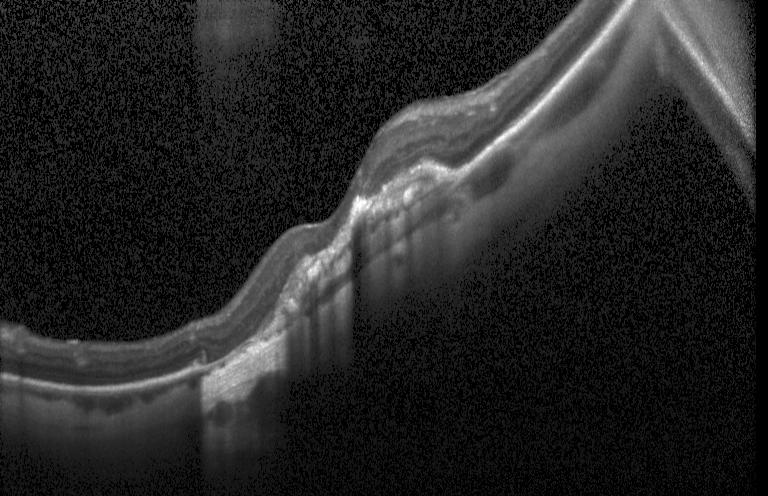
Finding: choroidal neovascularization (CNV).